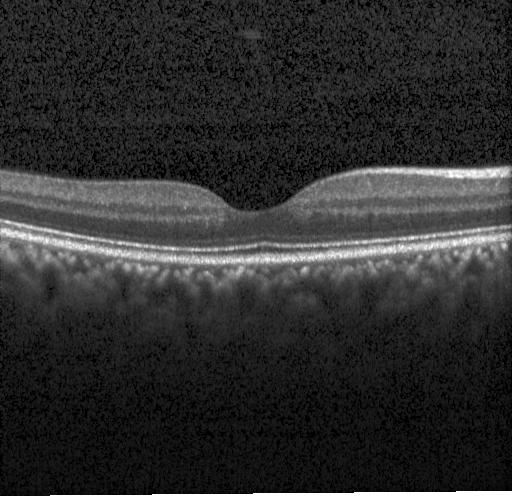 Heidelberg Spectralis. SD-OCT. Optical coherence tomography scan. Centered on the fovea. Finding: no choroidal neovascularization, diabetic macular edema, or drusen.